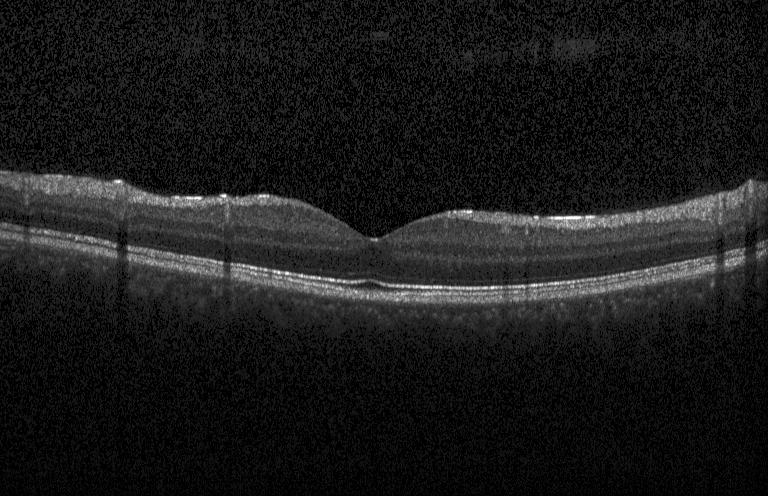
Macular OCT: no evidence of choroidal neovascularization, diabetic macular edema, or drusen.